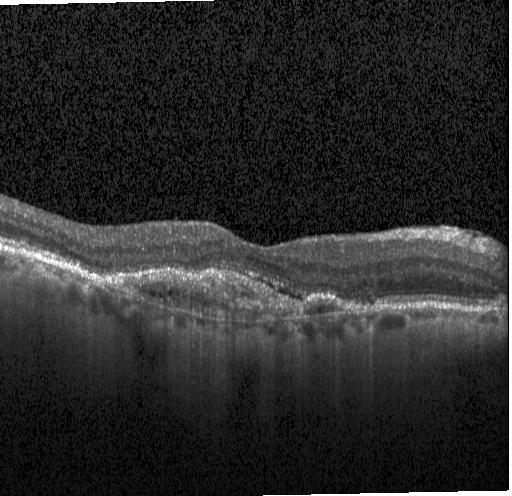 OCT finding: a choroidal neovascular membrane.